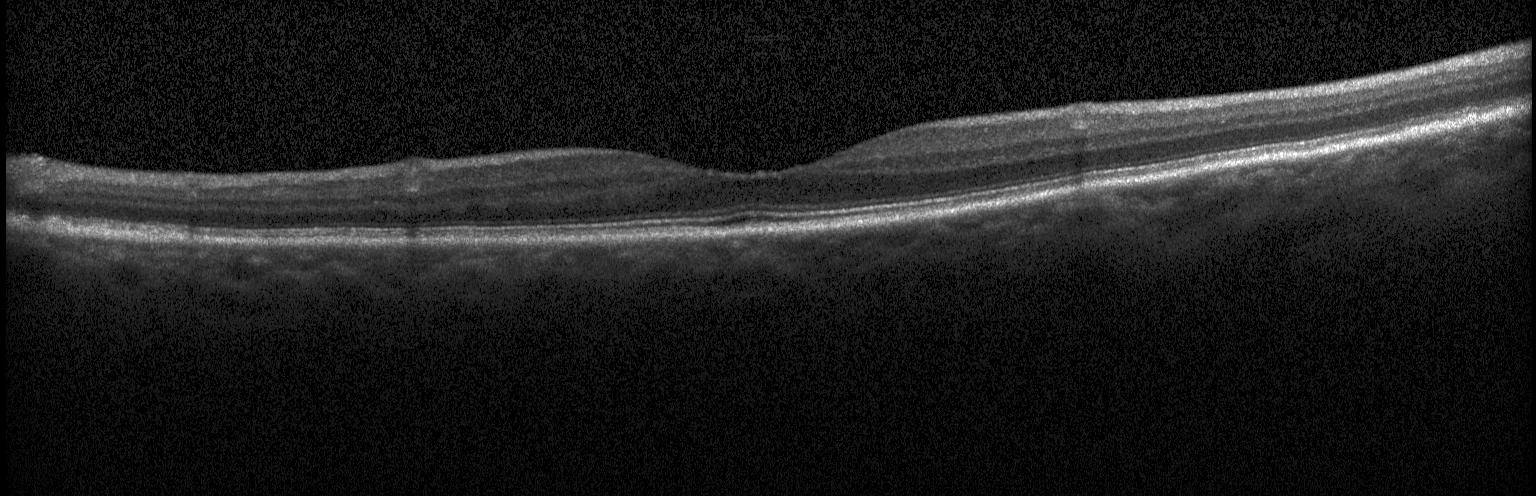 Optical coherence tomography scan; macular scan.
Assessment: no choroidal neovascularization, no diabetic macular edema, and no drusen.